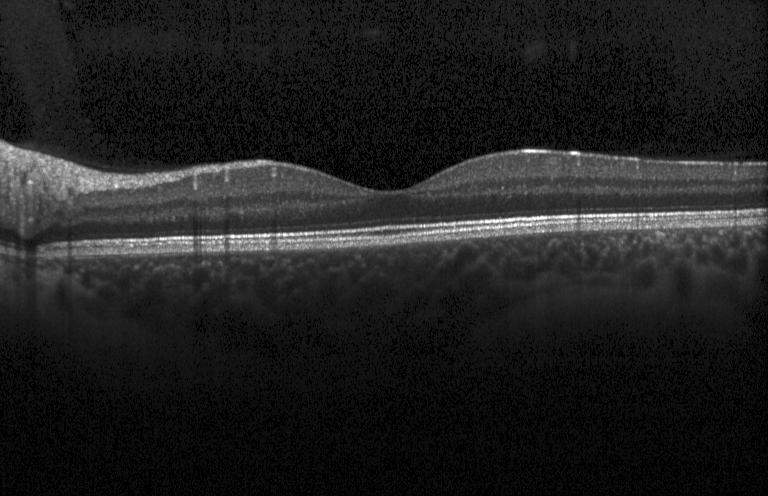 Retinal OCT B-scan. Heidelberg Spectralis OCT system. Spectral-domain optical coherence tomography. Macular scan — No evidence of choroidal neovascularization, diabetic macular edema, or drusen.